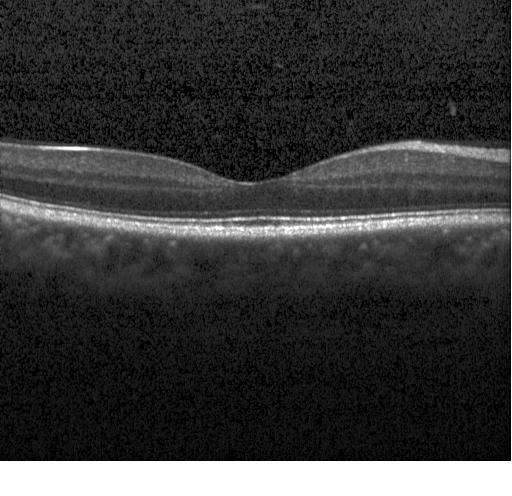 Optical coherence tomography scan — Diagnosis: no CNV, DME, or drusen.